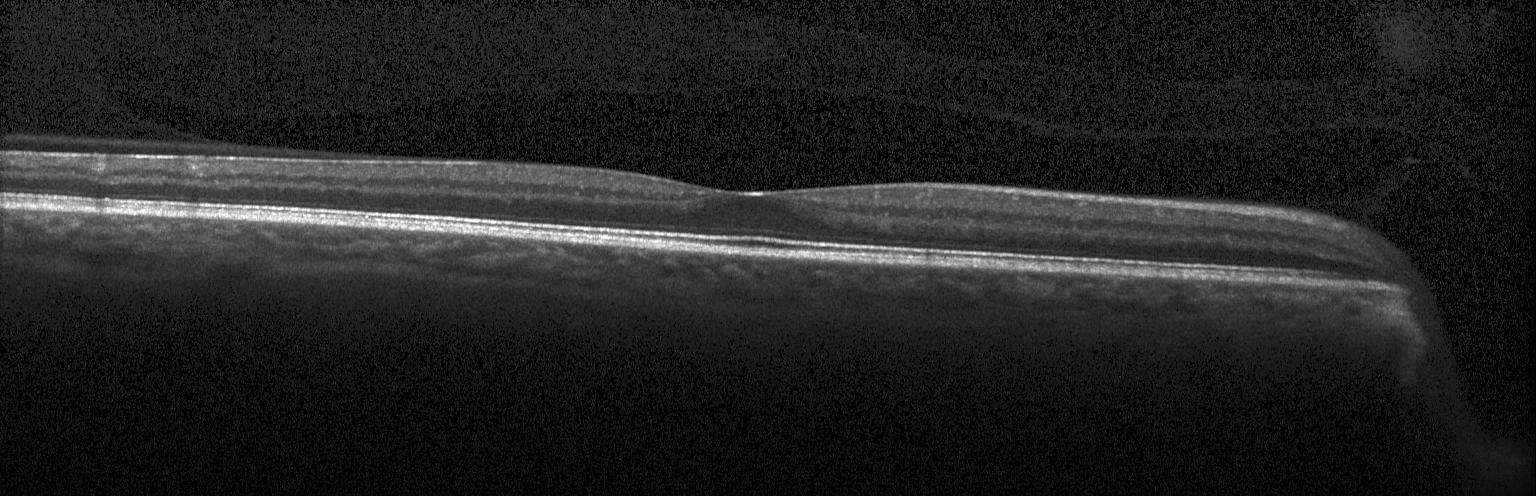 Finding: no evidence of choroidal neovascularization, diabetic macular edema, or drusen.